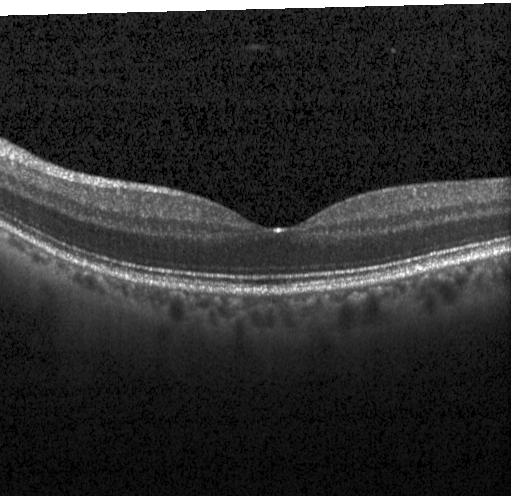
Spectral-domain OCT. Instrument: Heidelberg Spectralis. Through the macula. Retinal OCT B-scan. Diagnosis: no CNV, DME, or drusen.